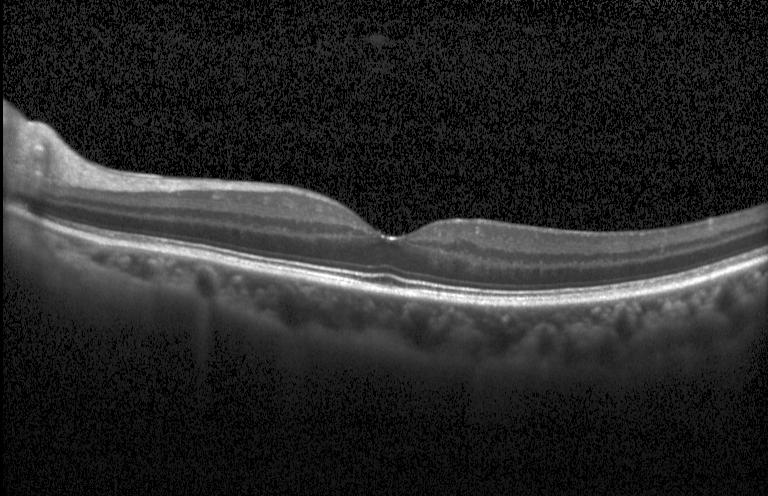 Macular OCT demonstrating no choroidal neovascularization, no diabetic macular edema, and no drusen.